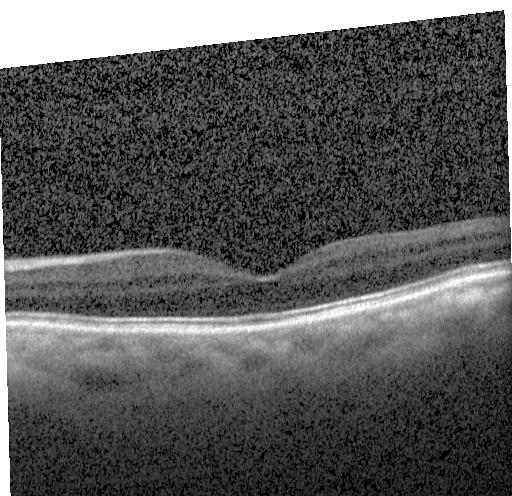

OCT B-scan. Acquired on a Heidelberg Spectralis.
The scan shows no choroidal neovascularization, diabetic macular edema, or drusen.